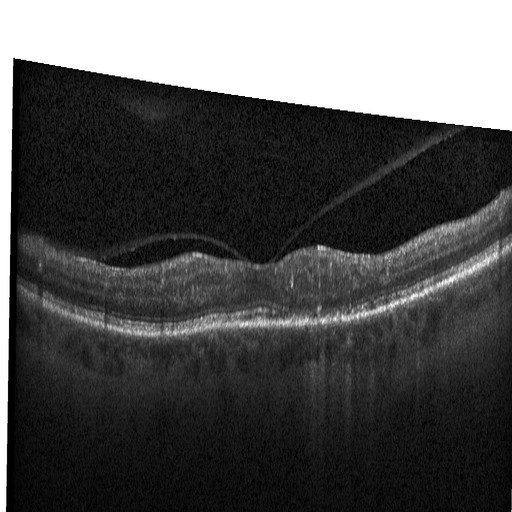 Dx: diabetic macular edema (DME).